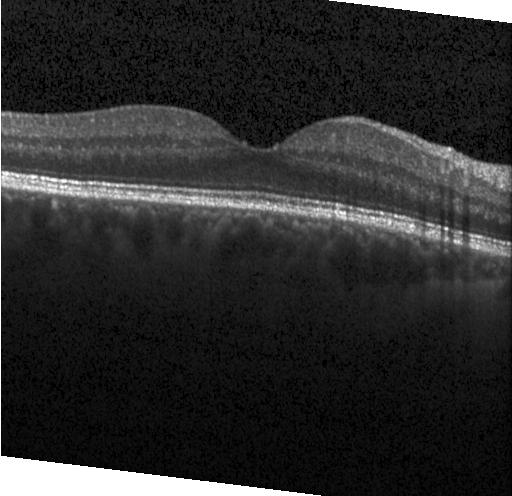
Impression: neither CNV, DME, nor drusen.